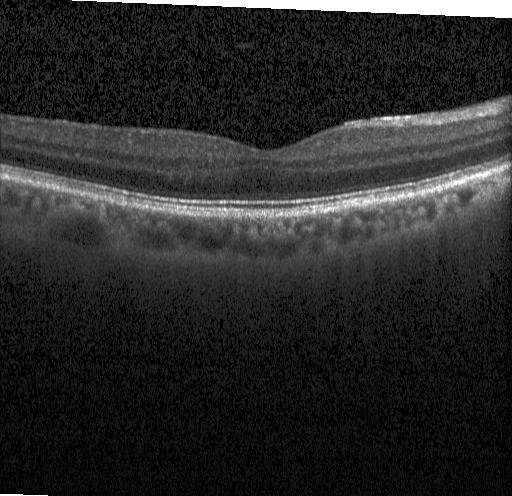
Through the macula. OCT B-scan. Spectral-domain optical coherence tomography. Heidelberg Spectralis — Dx: no evidence of choroidal neovascularization, diabetic macular edema, or drusen.